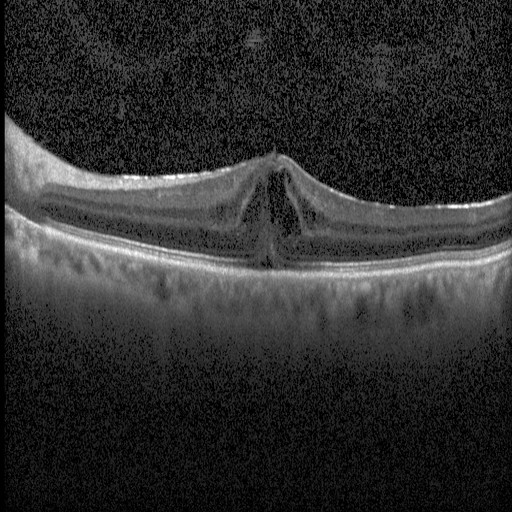

Macular OCT: DME.